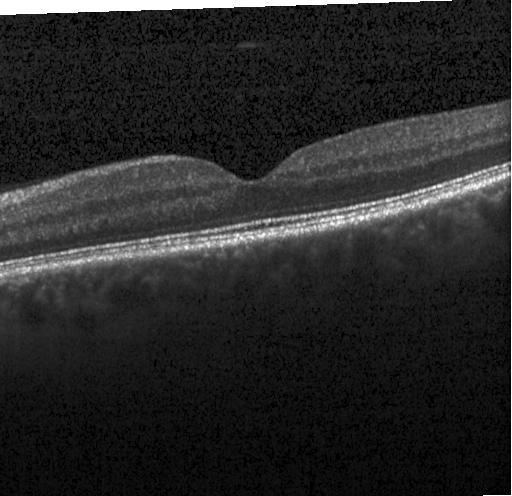
Macular scan · Heidelberg Spectralis · retinal OCT cross-section.
This B-scan demonstrates neither choroidal neovascularization, diabetic macular edema, nor drusen.